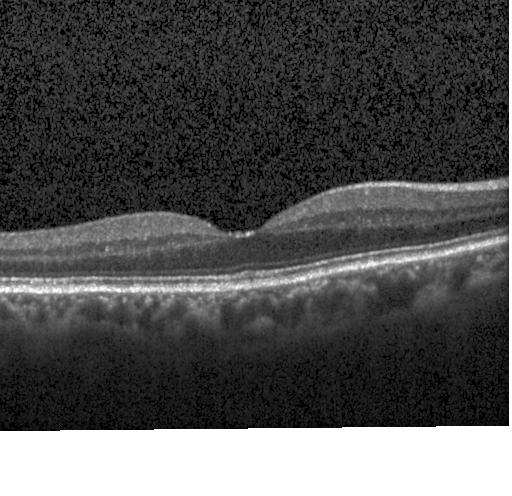

Macular OCT: neither choroidal neovascularization, diabetic macular edema, nor drusen.